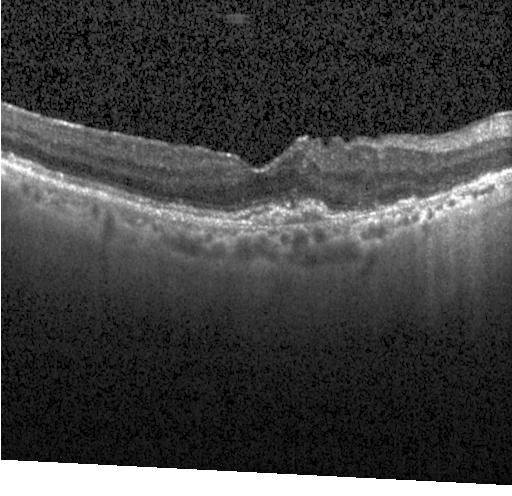 Optical coherence tomography B-scan; centered on the fovea
This B-scan demonstrates choroidal neovascularization.